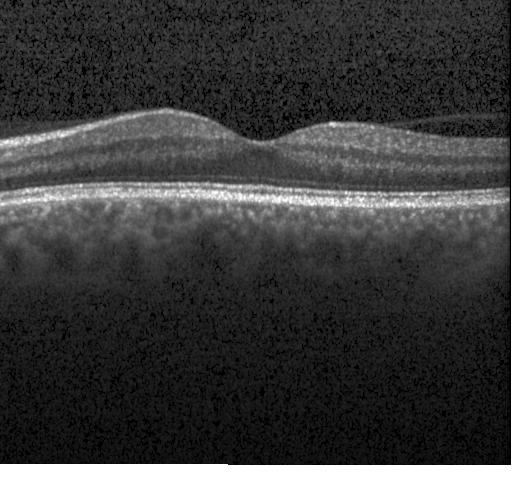 Assessment: no choroidal neovascularization, diabetic macular edema, or drusen.